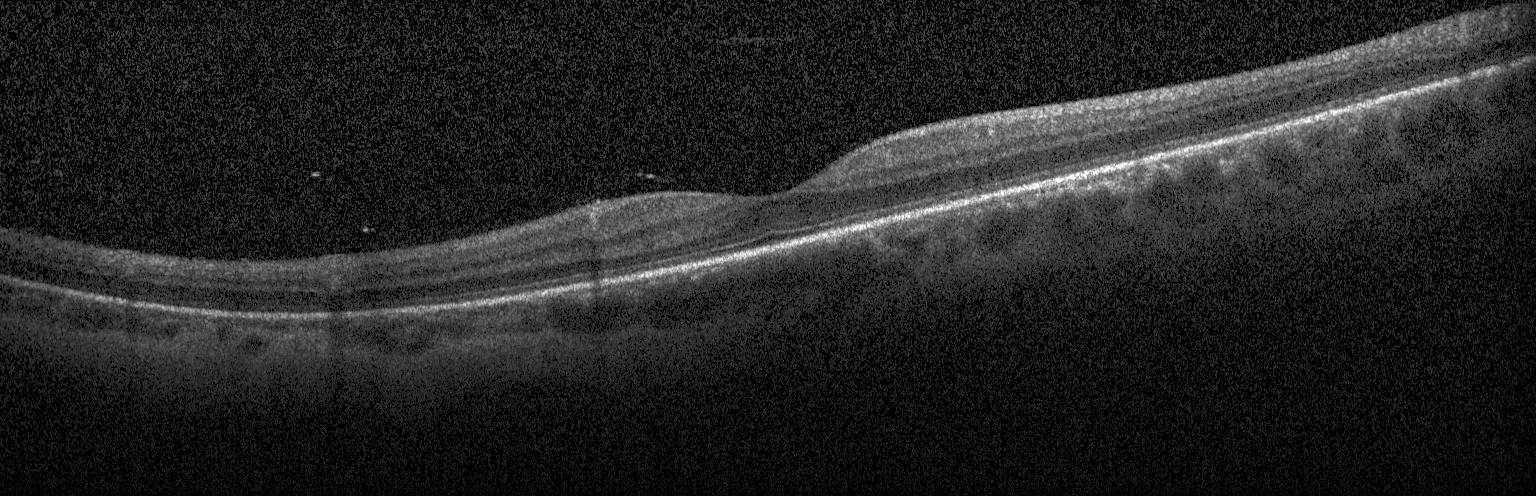 Assessment: neither choroidal neovascularization, diabetic macular edema, nor drusen.